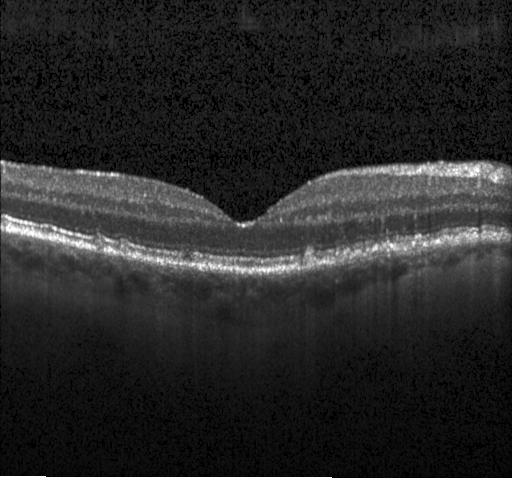

OCT scan showing drusen.